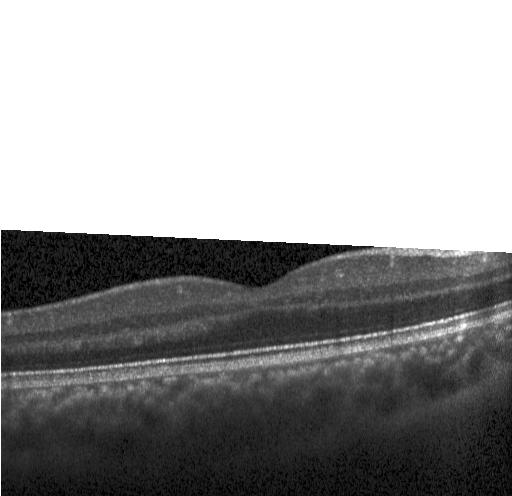
Finding: no choroidal neovascularization, diabetic macular edema, or drusen.